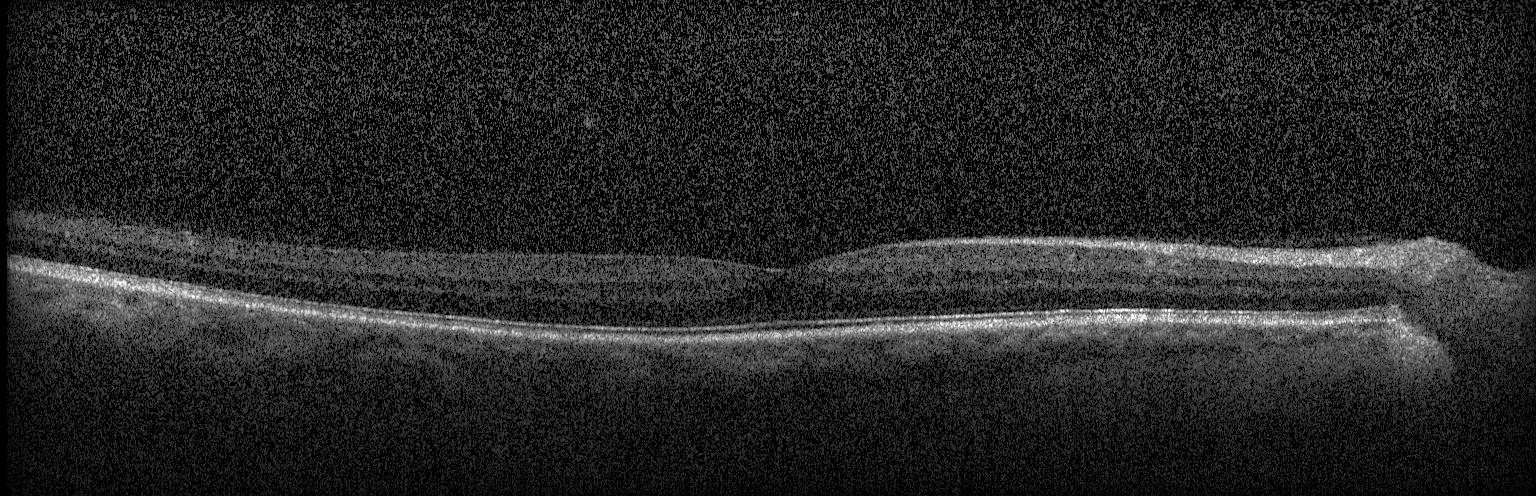
Spectral-domain optical coherence tomography; optical coherence tomography scan. The scan shows no choroidal neovascularization, no diabetic macular edema, and no drusen.